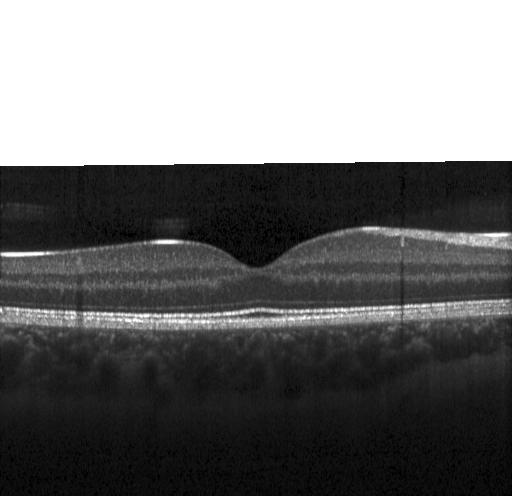 Retinal OCT cross-section. This B-scan demonstrates no choroidal neovascularization, diabetic macular edema, or drusen.